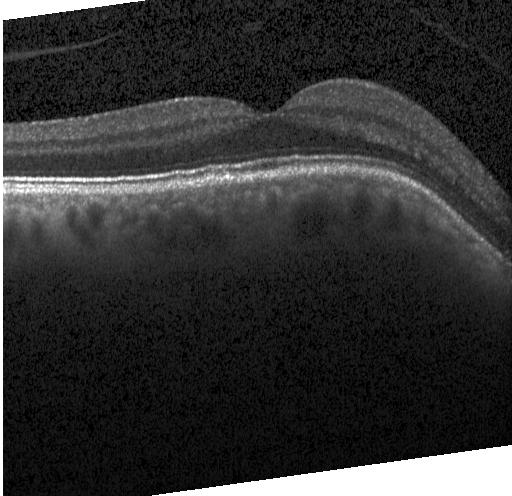
Retinal OCT cross-section. Horizontal scan through the fovea
The scan shows no choroidal neovascularization, no diabetic macular edema, and no drusen.